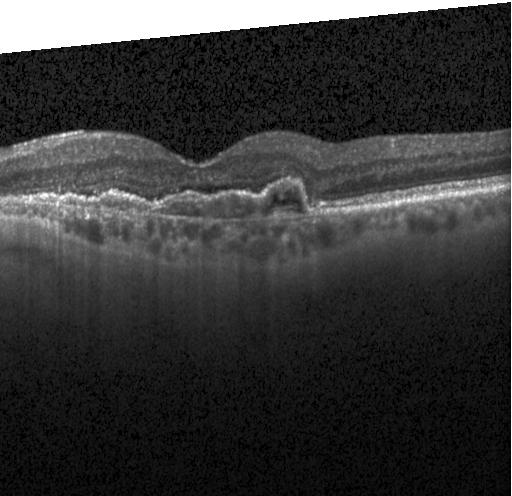

Spectral-domain optical coherence tomography. Heidelberg Spectralis OCT system. Macular scan. Retinal OCT B-scan.
Finding: choroidal neovascularization (CNV).